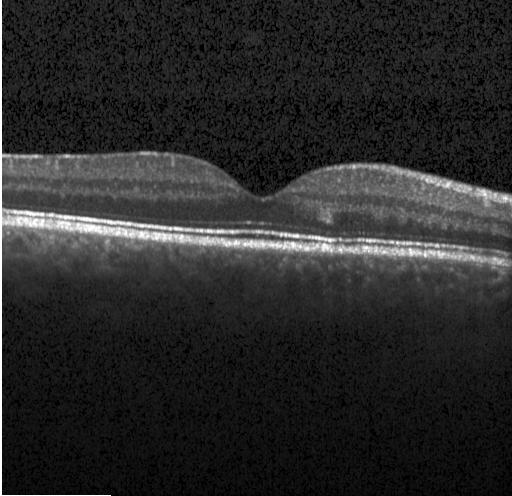

Impression: neither CNV, DME, nor drusen.